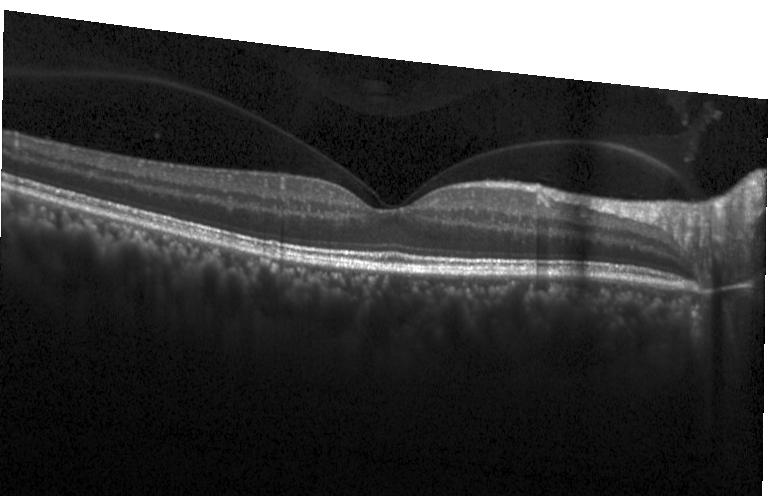

SD-OCT; retinal OCT B-scan; horizontal scan through the fovea. Diagnosis: no evidence of choroidal neovascularization, diabetic macular edema, or drusen.